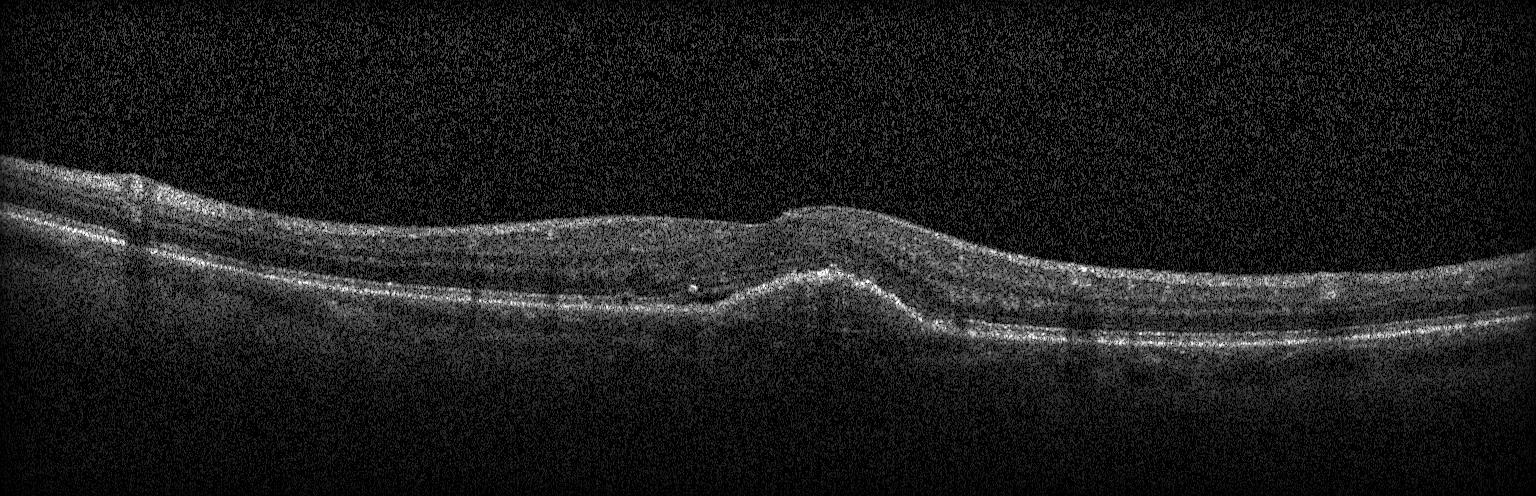
OCT line scan; through the macula
Impression: CNV.